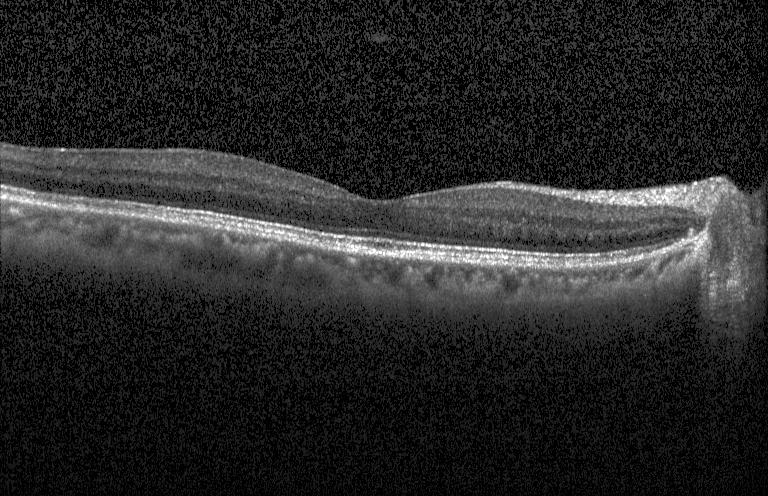

Through the macula. Spectral-domain optical coherence tomography. Heidelberg Spectralis OCT system. Retinal OCT cross-section. Assessment: no evidence of choroidal neovascularization, diabetic macular edema, or drusen.